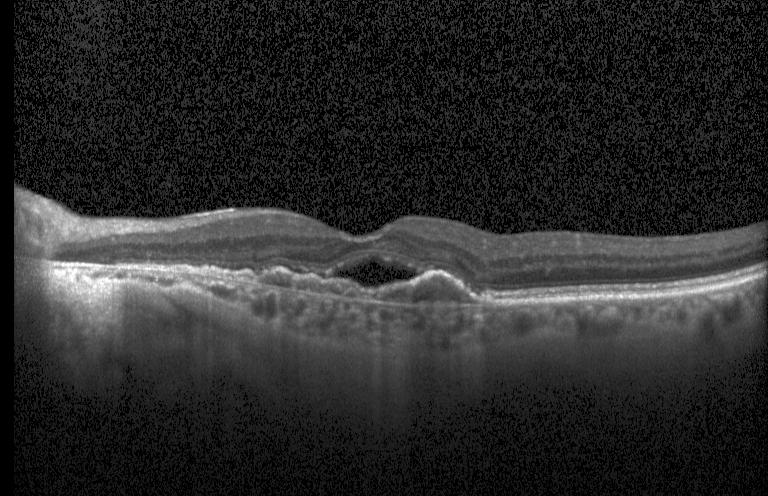

Optical coherence tomography scan
Assessment: a choroidal neovascular membrane.